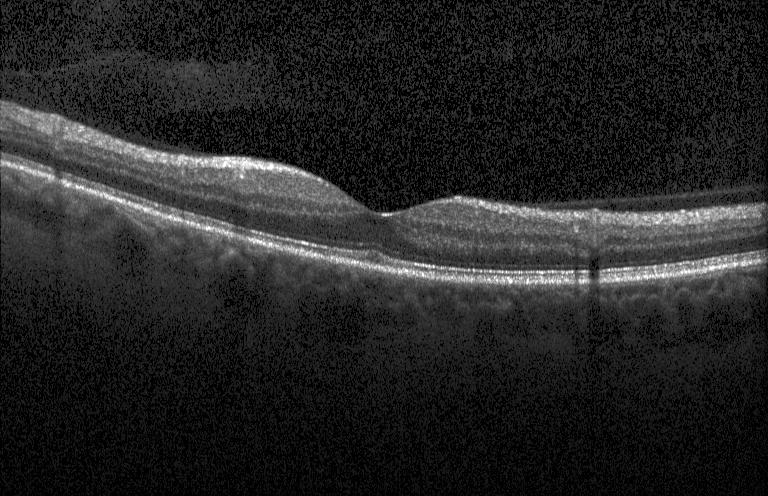
Impression: no choroidal neovascularization, diabetic macular edema, or drusen.